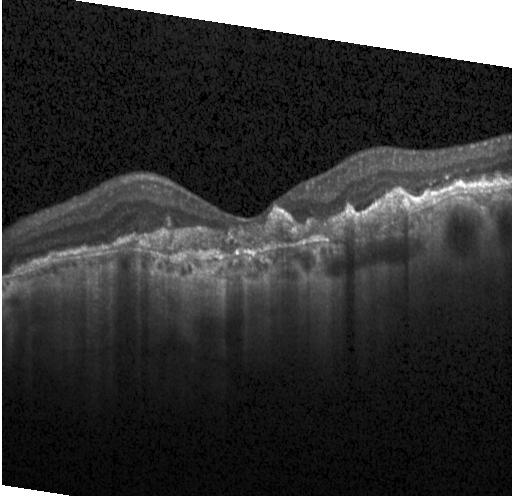

OCT finding: choroidal neovascularization (CNV).